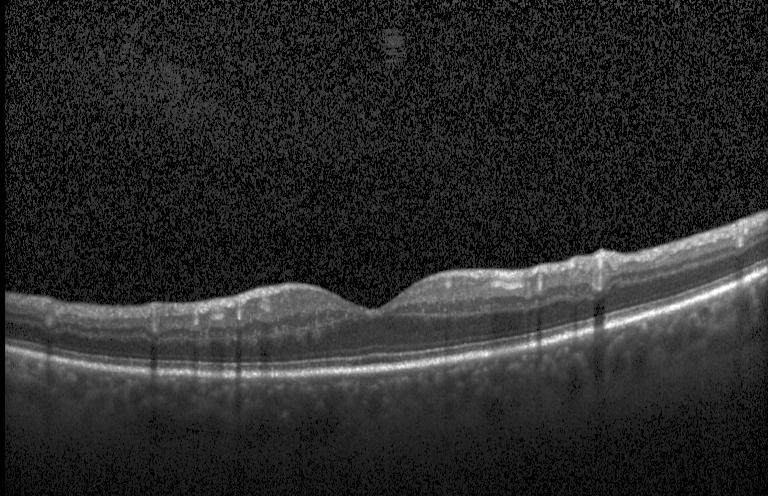

Neither choroidal neovascularization, diabetic macular edema, nor drusen.